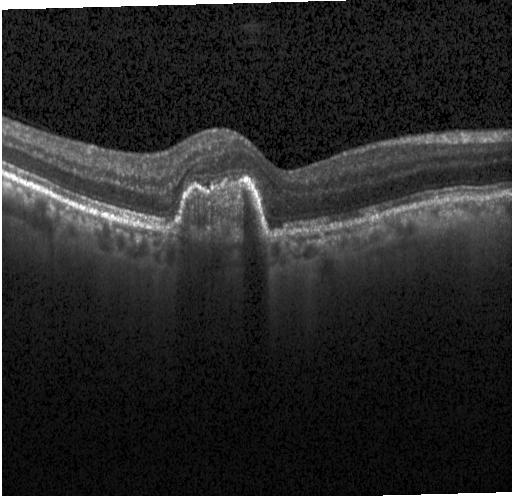
Finding: a choroidal neovascular membrane.